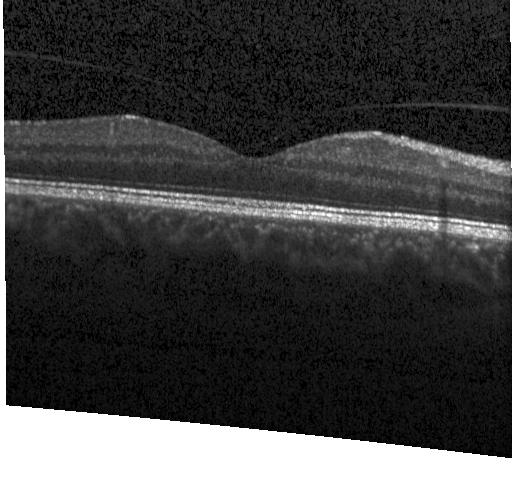

Finding: no evidence of choroidal neovascularization, diabetic macular edema, or drusen.